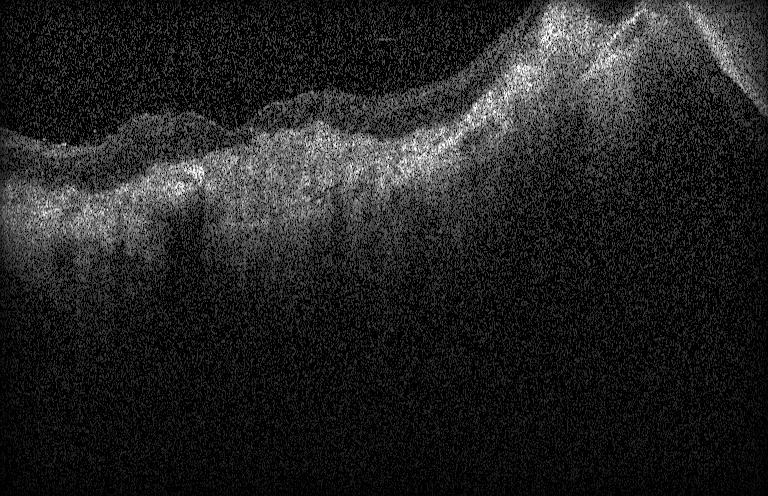
Optical coherence tomography B-scan. Macular OCT: choroidal neovascularization.